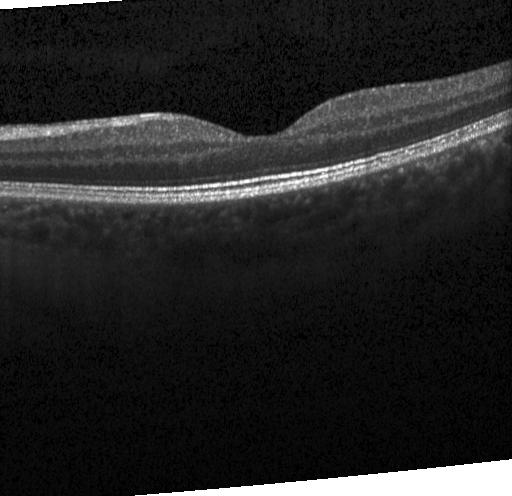 OCT B-scan showing neither choroidal neovascularization, diabetic macular edema, nor drusen.